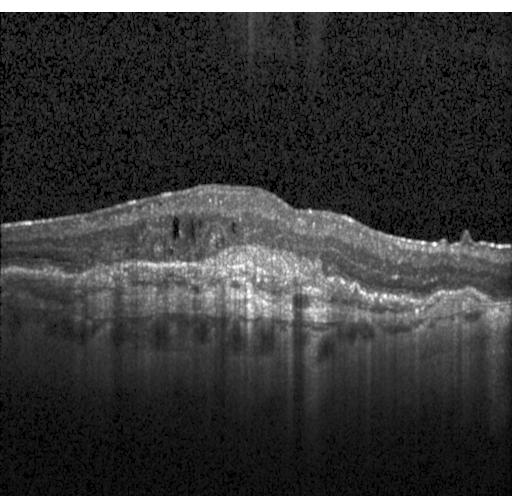 Choroidal neovascularization.